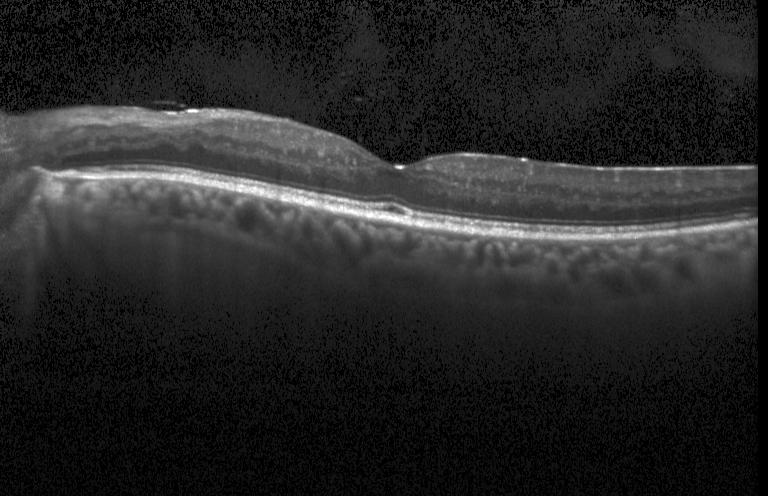

OCT finding: no CNV, no DME, and no drusen.